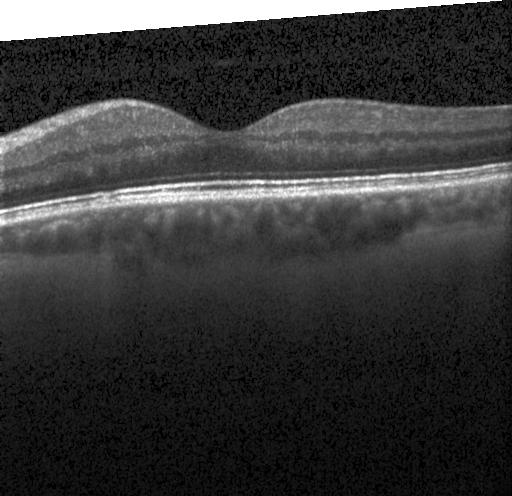
Retinal OCT cross-section.
The scan shows neither choroidal neovascularization, diabetic macular edema, nor drusen.